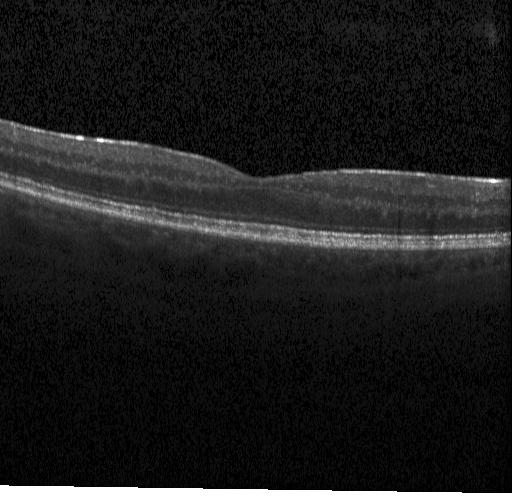 Heidelberg Spectralis. OCT B-scan. Spectral-domain OCT. Centered on the fovea
The scan shows no choroidal neovascularization, diabetic macular edema, or drusen.